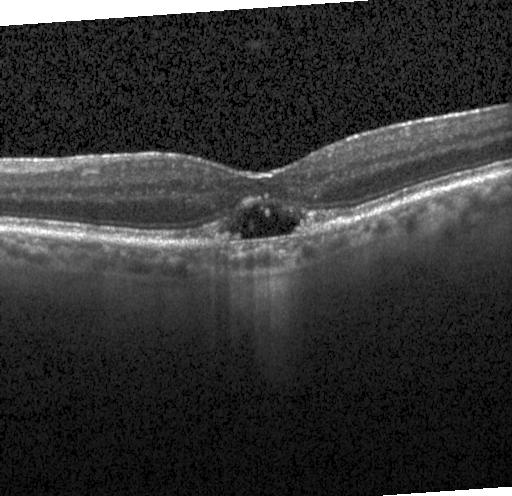 Finding: CNV.